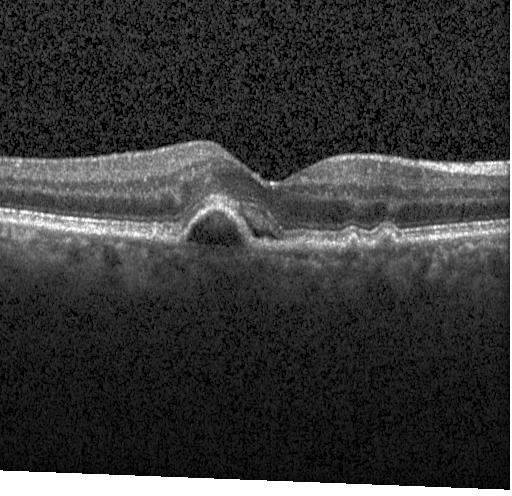
SD-OCT; optical coherence tomography scan. Assessment: a choroidal neovascular membrane.